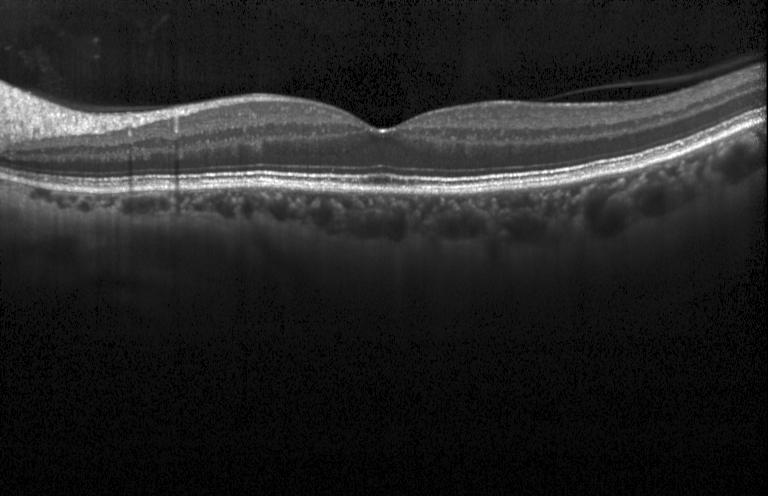 Optical coherence tomography scan; spectral-domain OCT; centered on the fovea; Heidelberg Spectralis — Diagnosis: no evidence of CNV, DME, or drusen.